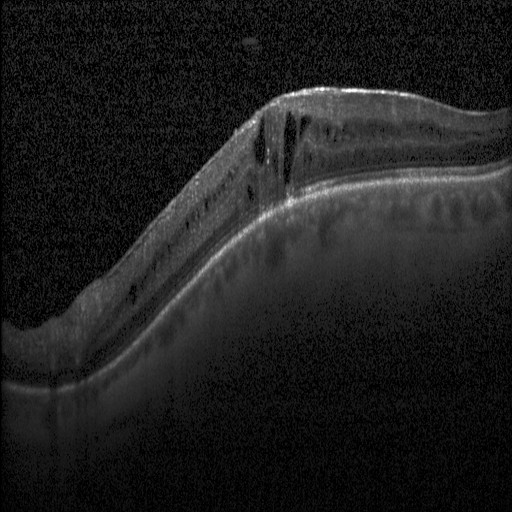

OCT B-scan. Spectral-domain optical coherence tomography. Through the macula. Instrument: Heidelberg Spectralis
Finding: diabetic macular edema (DME).